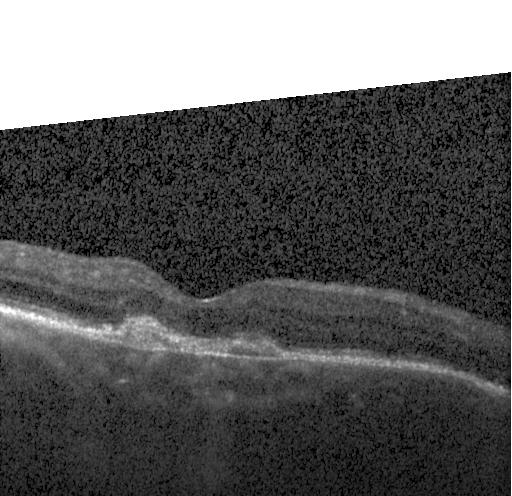 Macular OCT demonstrating CNV.